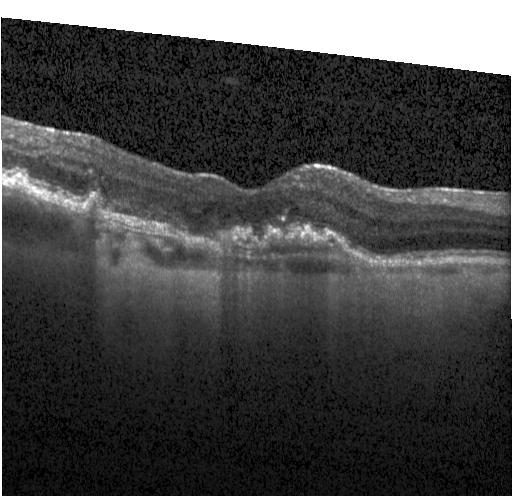

Macular OCT demonstrating CNV.